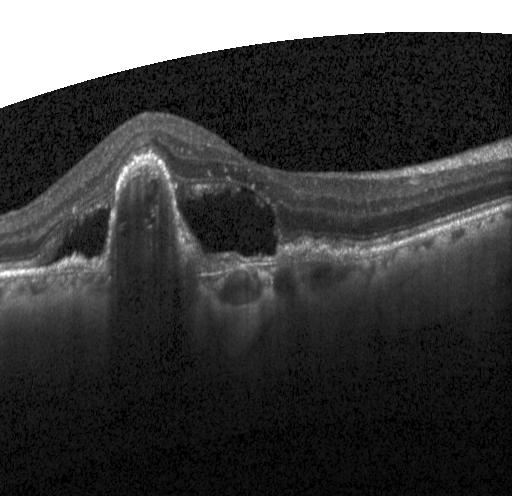

Spectral-domain OCT; macular scan; OCT B-scan. The scan shows CNV.